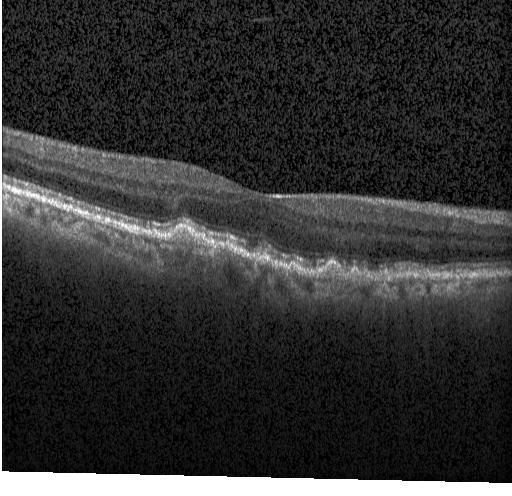
SD-OCT; macular scan; optical coherence tomography B-scan.
OCT finding: sub-RPE drusenoid deposits.